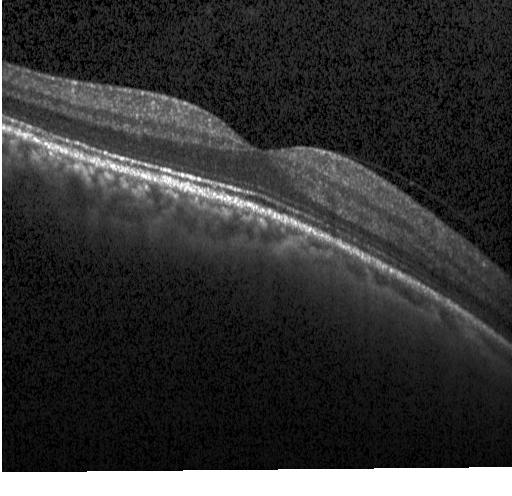

Finding: no evidence of CNV, DME, or drusen.